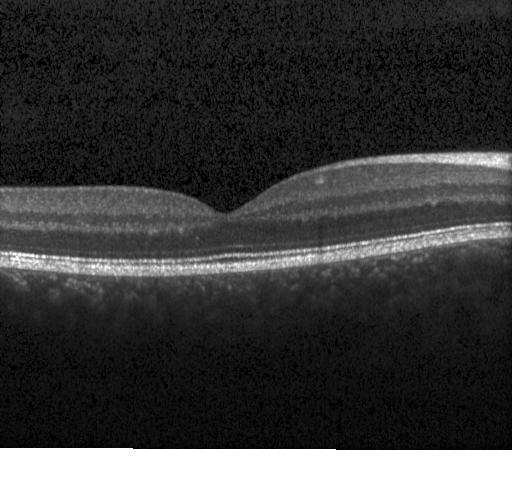 OCT B-scan, Heidelberg Spectralis. Impression: no CNV, no DME, and no drusen.